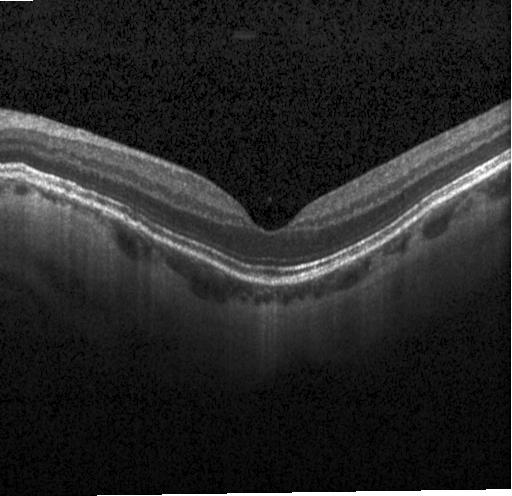

Optical coherence tomography scan.
Impression: no CNV, DME, or drusen.